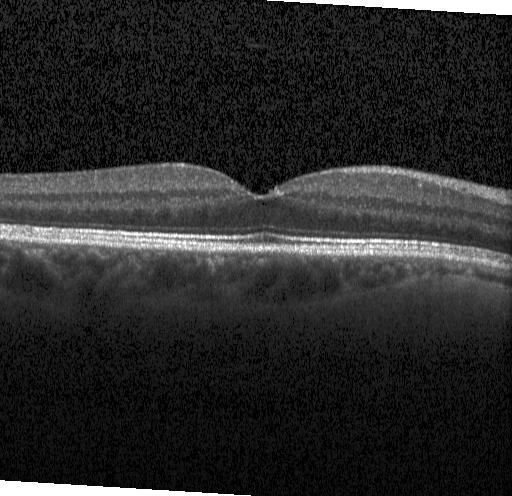 OCT line scan · SD-OCT.
This B-scan demonstrates no choroidal neovascularization, diabetic macular edema, or drusen.